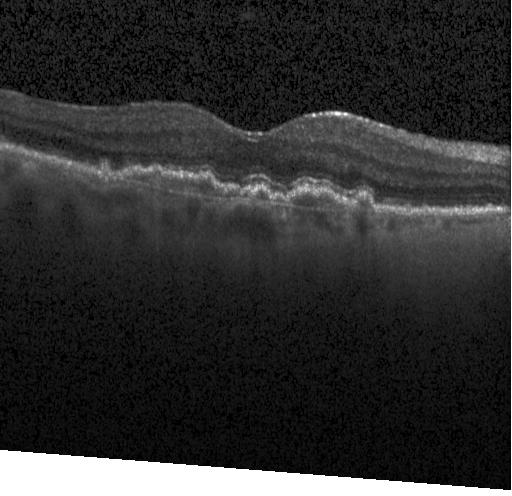
SD-OCT; optical coherence tomography scan; fovea-centered. Impression: a choroidal neovascular membrane.